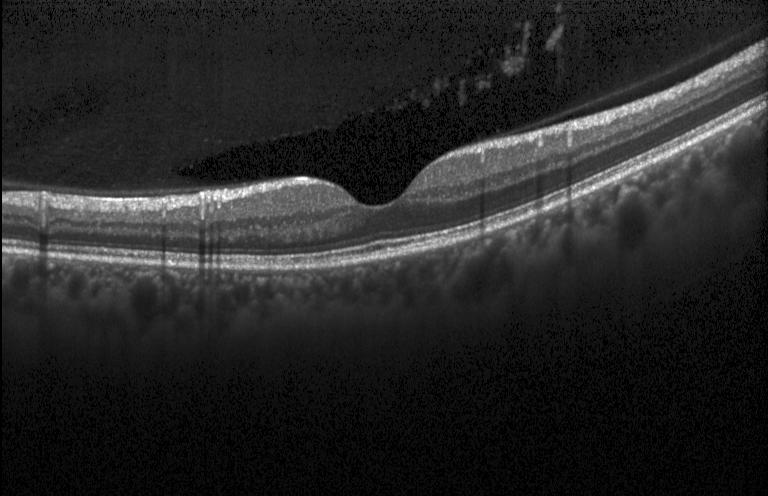
Finding: no evidence of CNV, DME, or drusen.